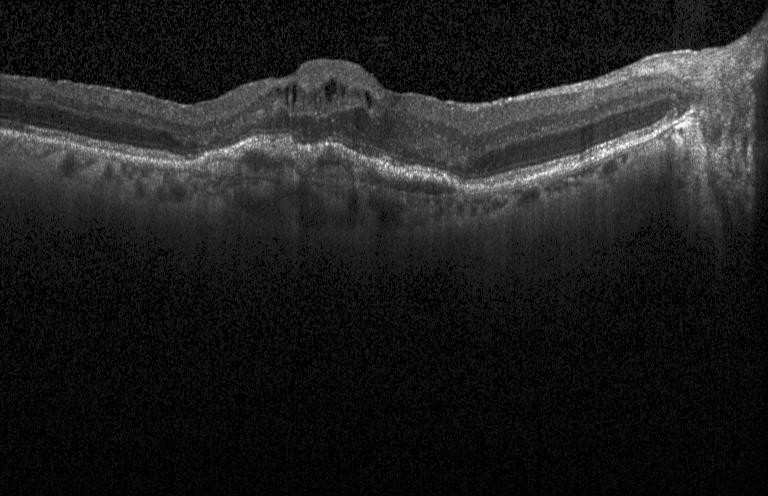
Assessment: a choroidal neovascular membrane.